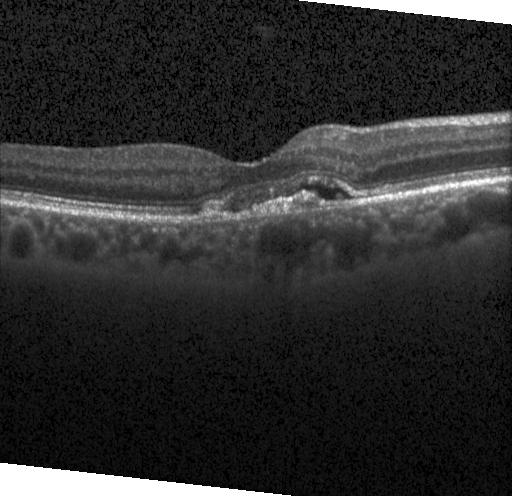
OCT B-scan.
Diagnosis: a choroidal neovascular membrane.